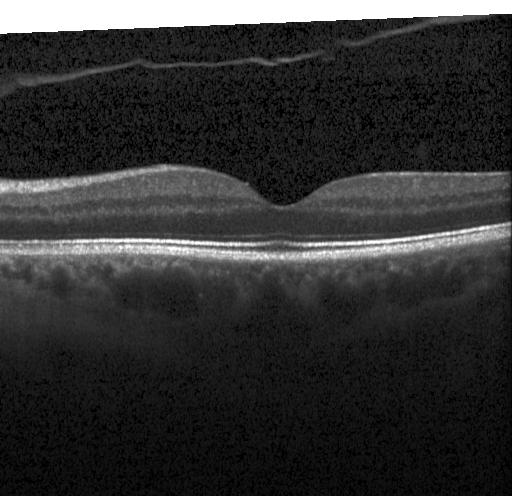

Assessment: no choroidal neovascularization, no diabetic macular edema, and no drusen.